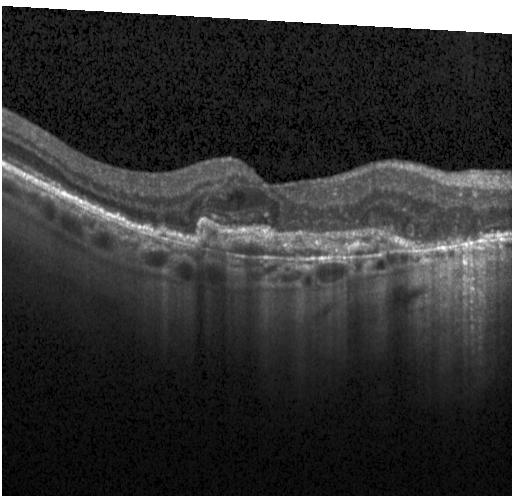

Through the macula, spectral-domain optical coherence tomography, OCT line scan, Heidelberg Spectralis — This B-scan demonstrates a choroidal neovascular membrane.